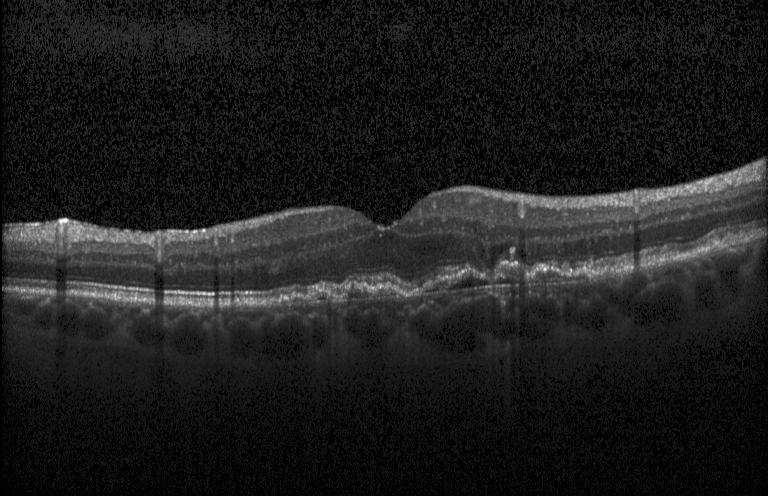

OCT line scan · spectral-domain optical coherence tomography · Heidelberg Spectralis OCT system · through the macula — Multiple drusen.